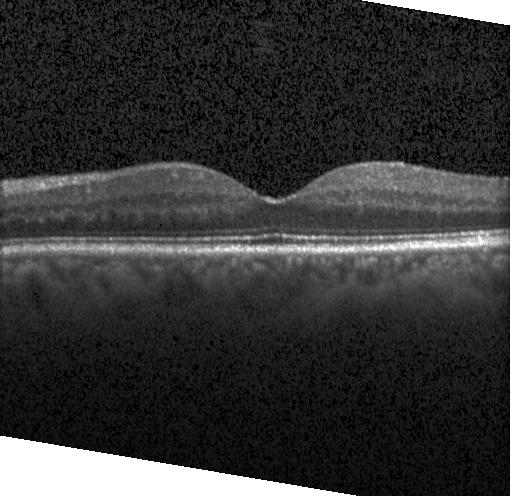

OCT line scan. Diagnosis: no choroidal neovascularization, no diabetic macular edema, and no drusen.